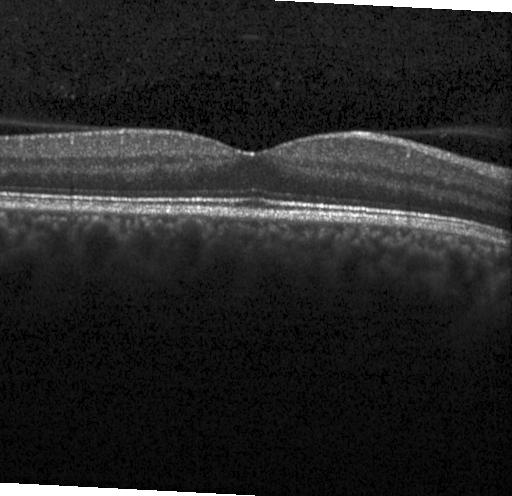

Retinal OCT cross-section showing no choroidal neovascularization, diabetic macular edema, or drusen.